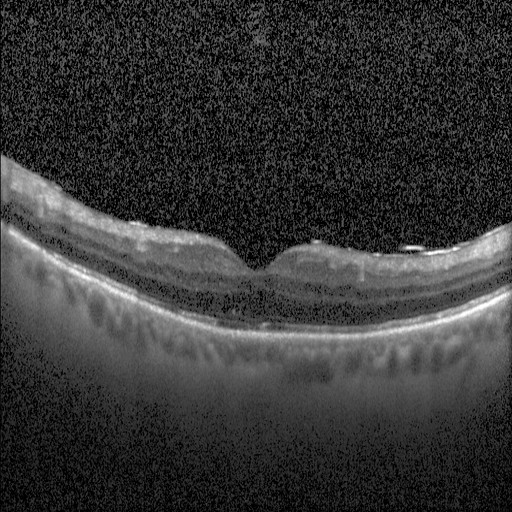

Instrument: Heidelberg Spectralis · retinal OCT cross-section · spectral-domain optical coherence tomography.
Finding: diabetic macular edema.